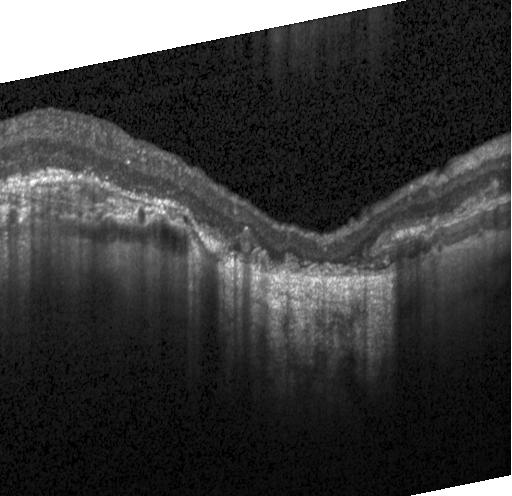
Assessment: choroidal neovascularization (CNV).